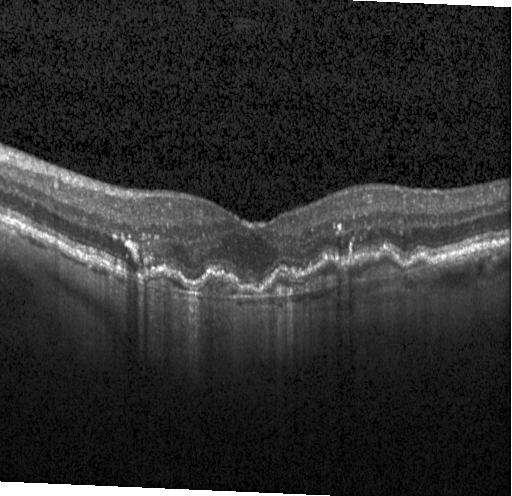

A choroidal neovascular membrane.